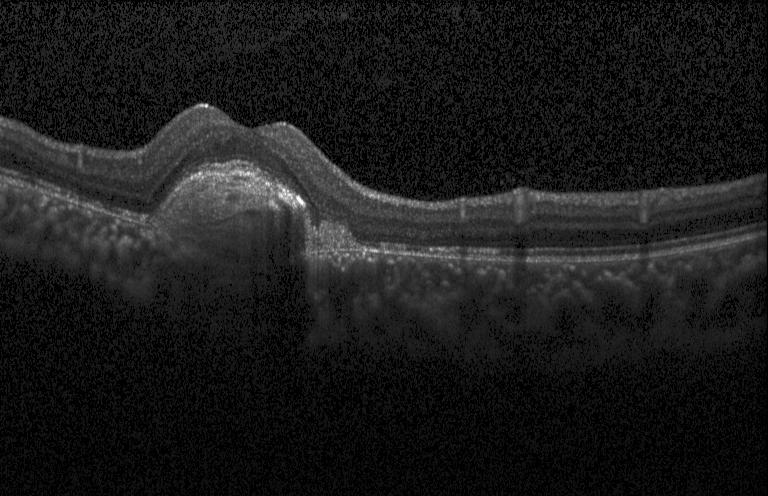
Macular OCT: a choroidal neovascular membrane.